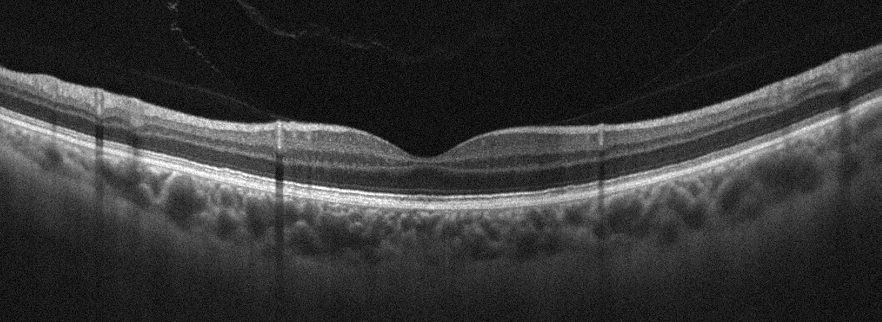

Retinal OCT cross-section; oculus dexter — Impression: no evidence of AMD, DME, ERM, RAO, RVO, or VID.